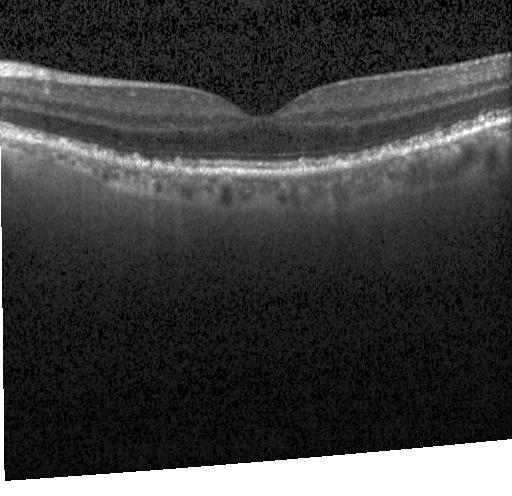 Diagnosis: drusen.